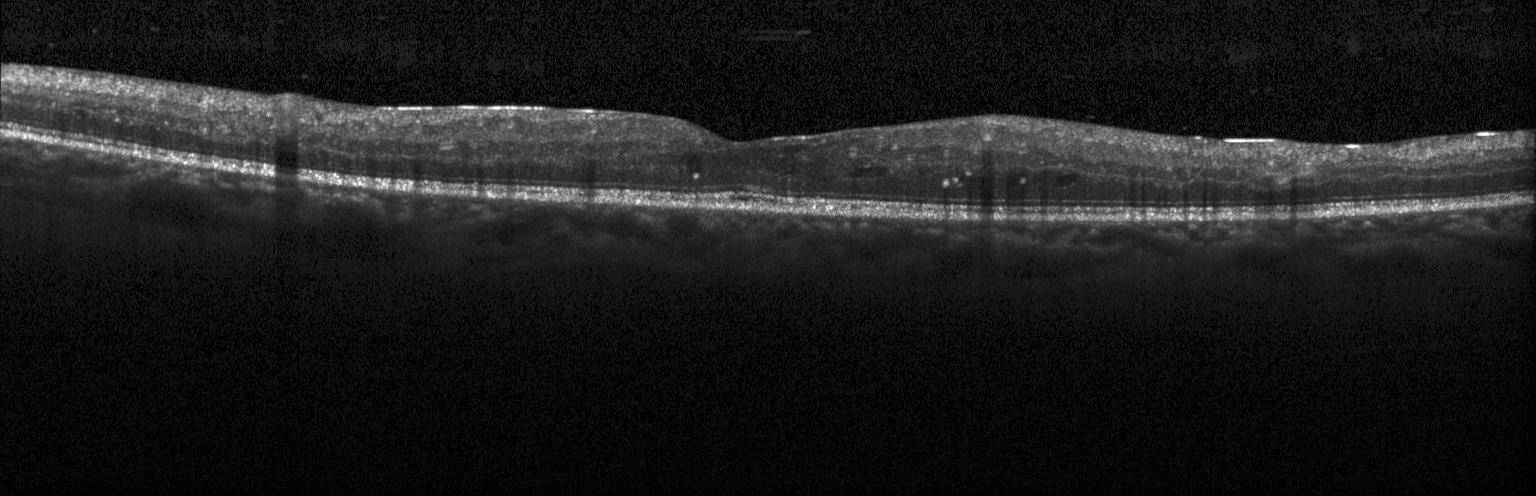 OCT line scan; instrument: Heidelberg Spectralis; through the macula; spectral-domain optical coherence tomography — This B-scan demonstrates diabetic macular edema (DME).